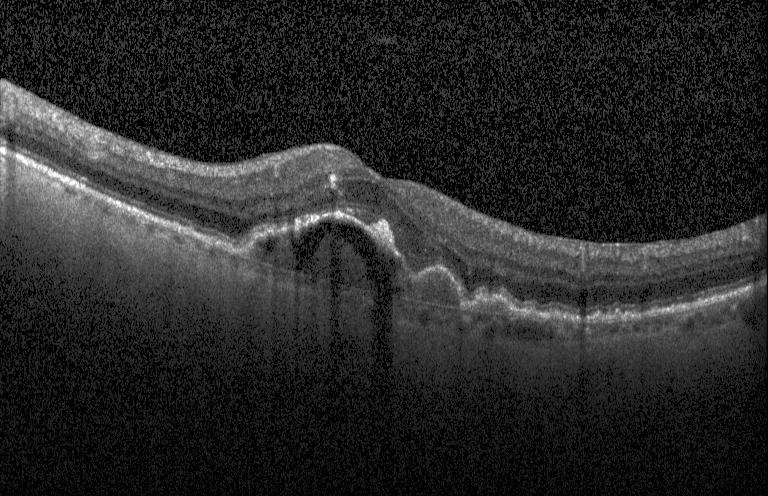 Retinal OCT B-scan.
A choroidal neovascular membrane.